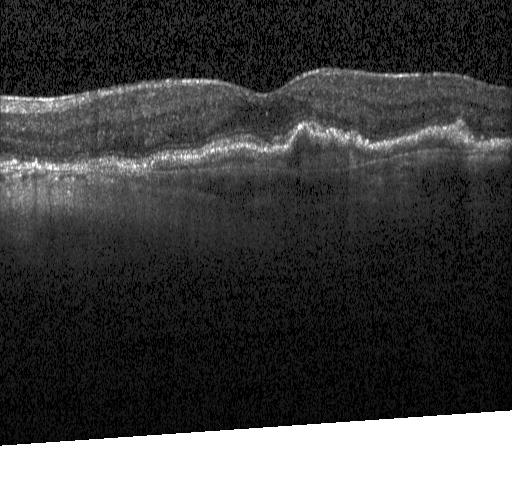
Centered on the fovea, optical coherence tomography scan.
Macular OCT: a choroidal neovascular membrane.